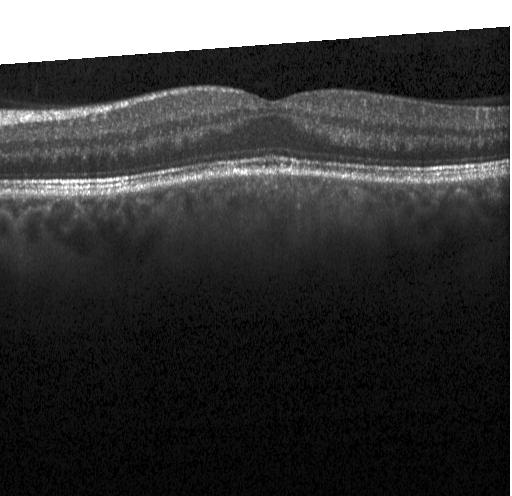
OCT line scan; spectral-domain OCT; fovea-centered.
Neither CNV, DME, nor drusen.